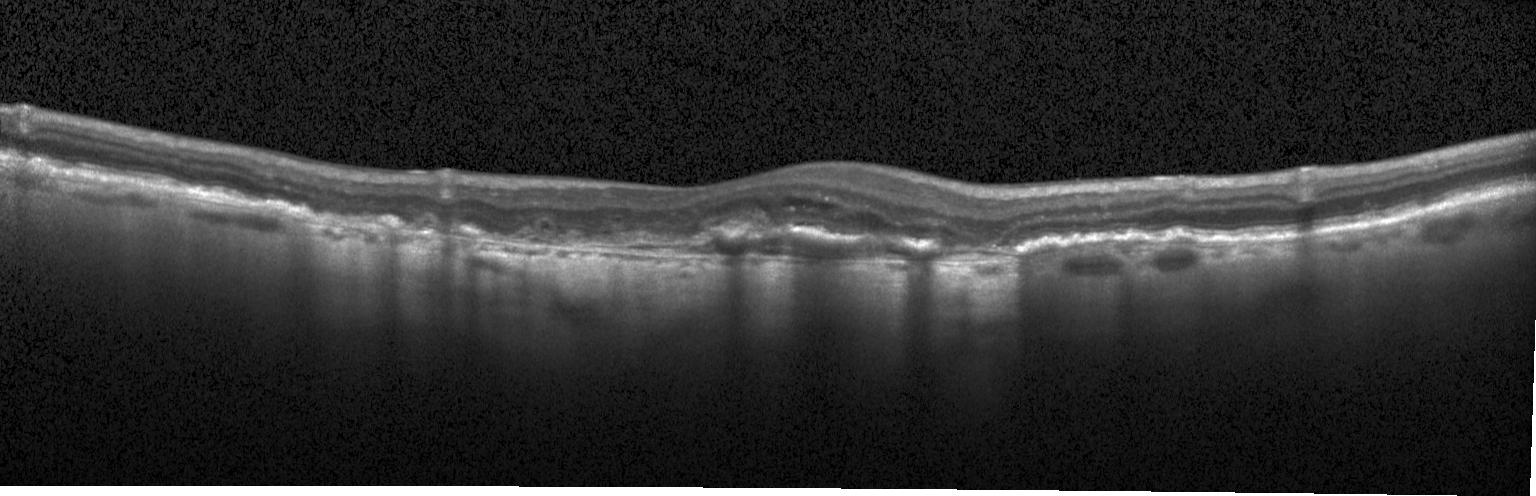

Acquired on a Heidelberg Spectralis, horizontal scan through the fovea, OCT B-scan — Macular OCT: a choroidal neovascular membrane.